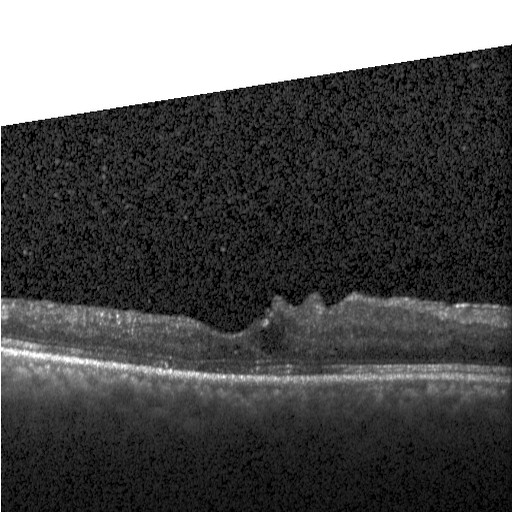
Through the macula; Heidelberg Spectralis OCT system; retinal OCT cross-section. Dx: DME.